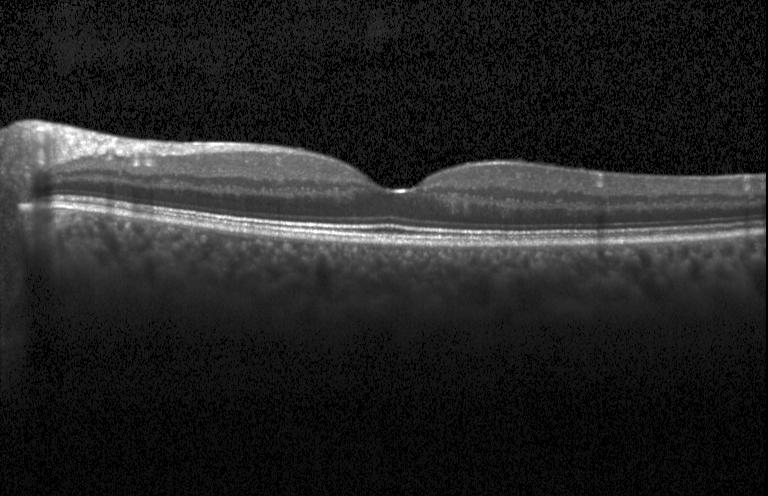
Acquired on a Heidelberg Spectralis, spectral-domain optical coherence tomography, retinal OCT cross-section — Impression: no choroidal neovascularization, no diabetic macular edema, and no drusen.